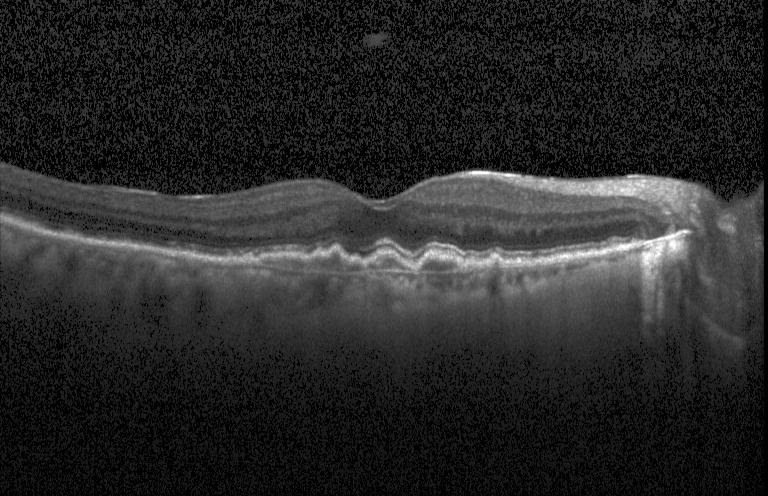 Diagnosis: choroidal neovascularization (CNV).